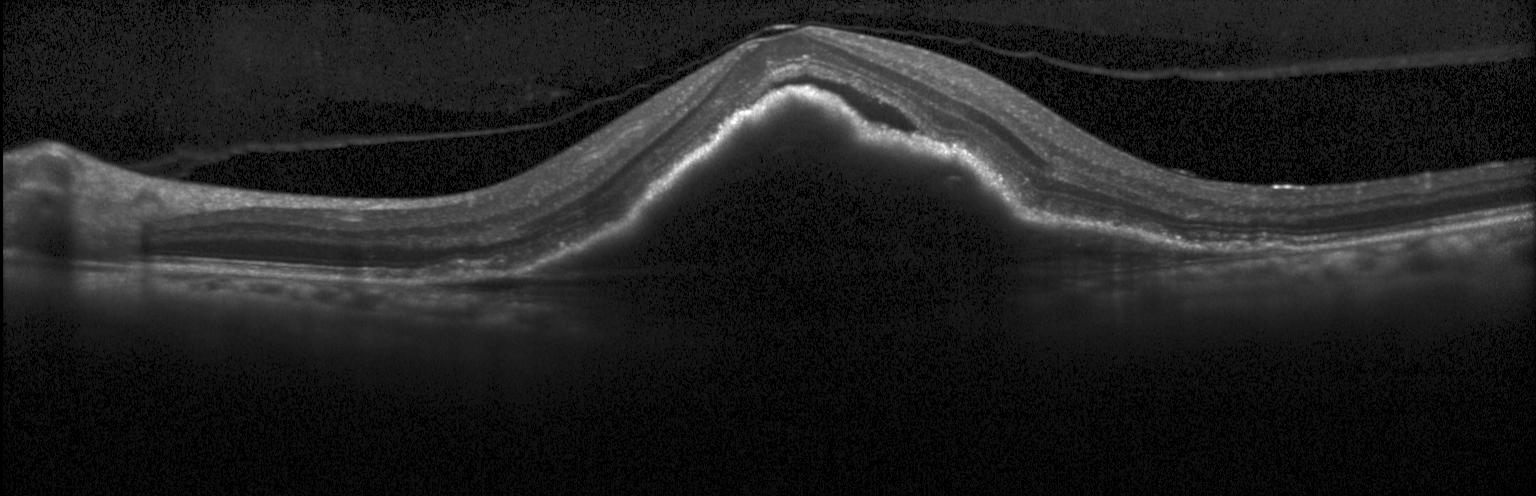 Macular OCT: a choroidal neovascular membrane.